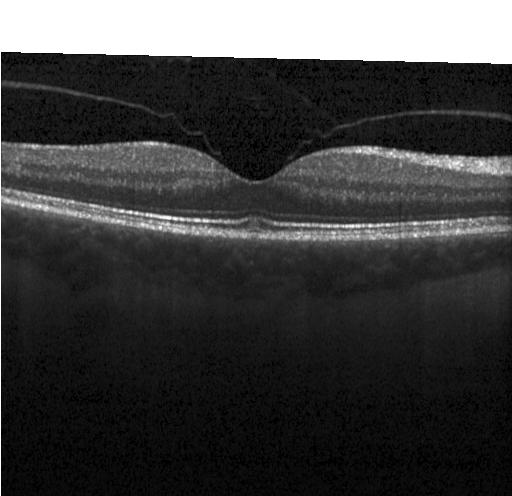
Impression: no evidence of choroidal neovascularization, diabetic macular edema, or drusen.